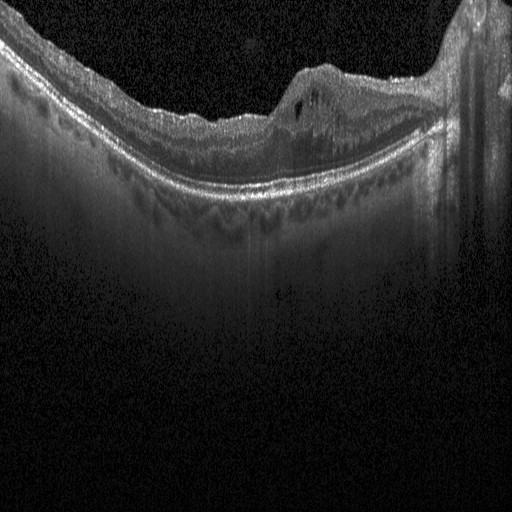

Diabetic macular edema.